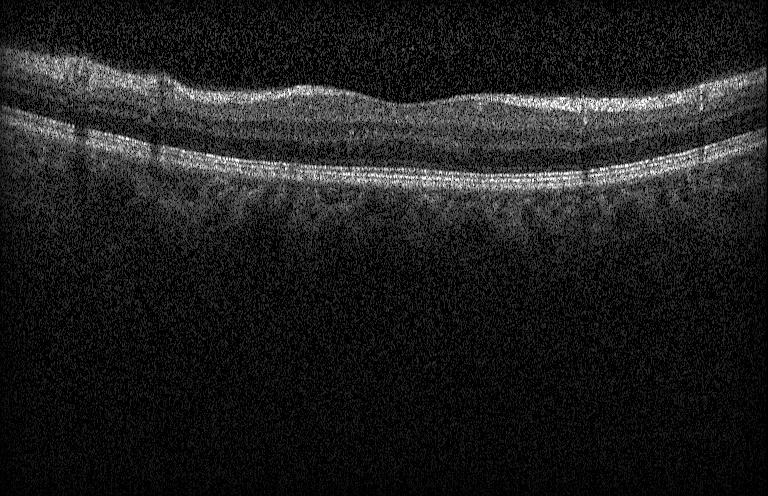
Instrument: Heidelberg Spectralis · fovea-centered · optical coherence tomography scan · SD-OCT. Finding: no choroidal neovascularization, diabetic macular edema, or drusen.